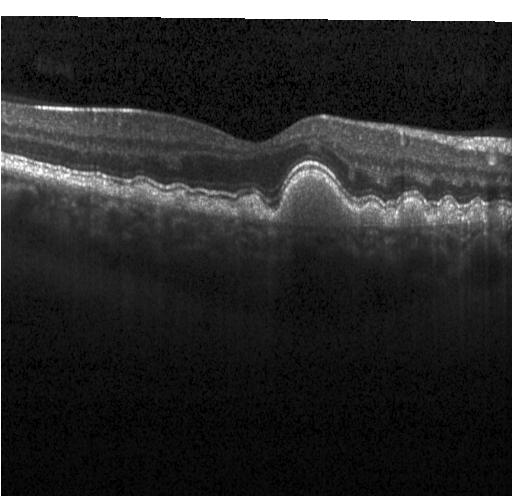

Retinal OCT cross-section, spectral-domain optical coherence tomography, through the macula. Impression: sub-RPE drusenoid deposits.